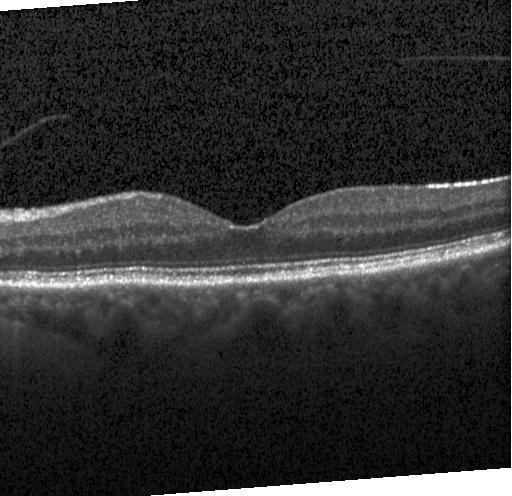 Finding: no evidence of choroidal neovascularization, diabetic macular edema, or drusen.